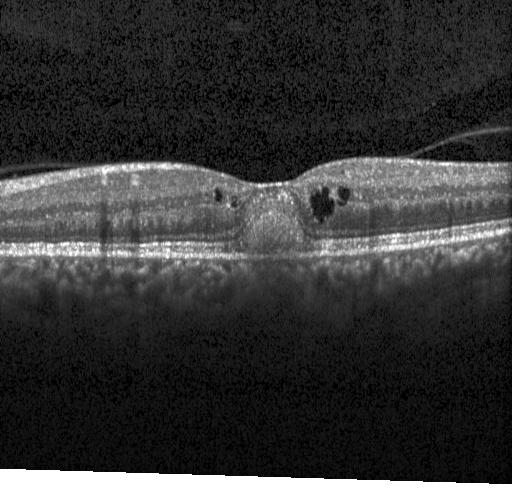
Macular scan; OCT line scan; spectral-domain optical coherence tomography
Impression: CNV.